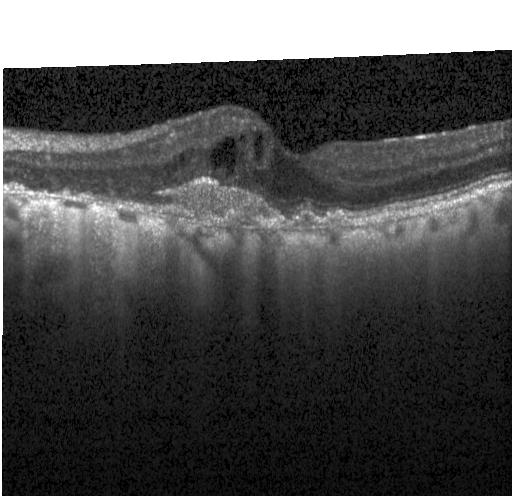

Diagnosis: a choroidal neovascular membrane.